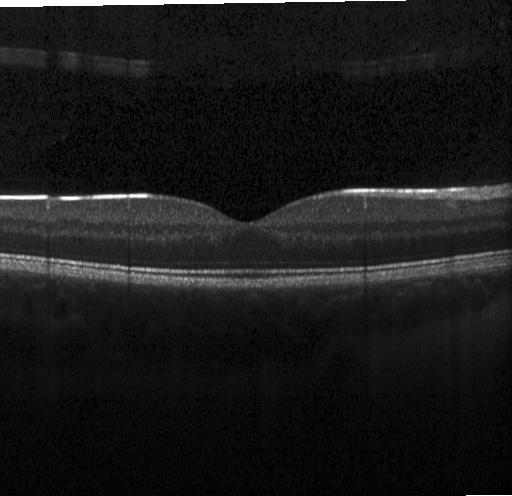
Fovea-centered. Spectral-domain OCT. Instrument: Heidelberg Spectralis. Retinal OCT cross-section
Diagnosis: no evidence of choroidal neovascularization, diabetic macular edema, or drusen.